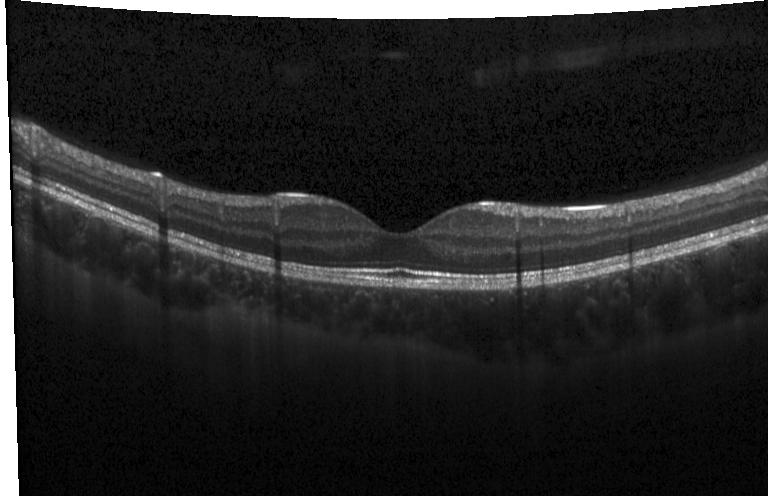 Horizontal scan through the fovea. Optical coherence tomography B-scan
Assessment: no evidence of choroidal neovascularization, diabetic macular edema, or drusen.